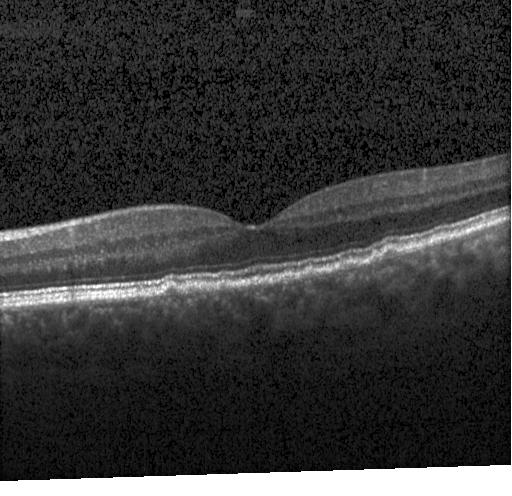 Spectral-domain optical coherence tomography · instrument: Heidelberg Spectralis · OCT line scan · through the macula — The scan shows multiple drusen.